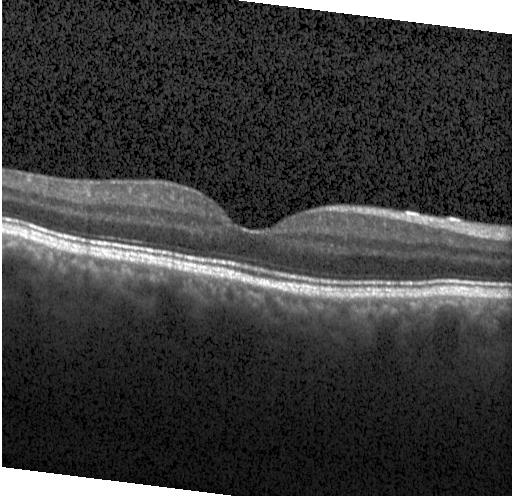
SD-OCT. OCT B-scan. Instrument: Heidelberg Spectralis.
Diagnosis: no choroidal neovascularization, no diabetic macular edema, and no drusen.